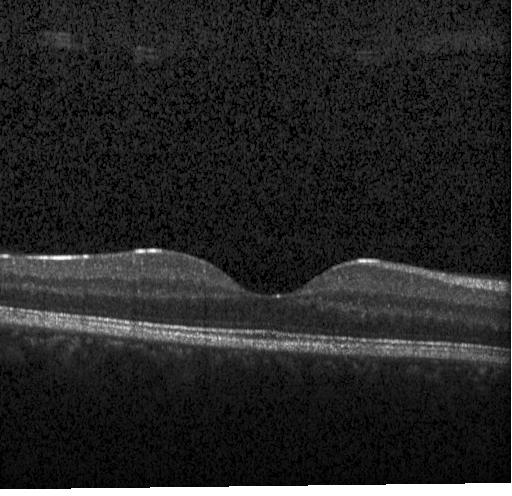

Finding: no choroidal neovascularization, diabetic macular edema, or drusen.